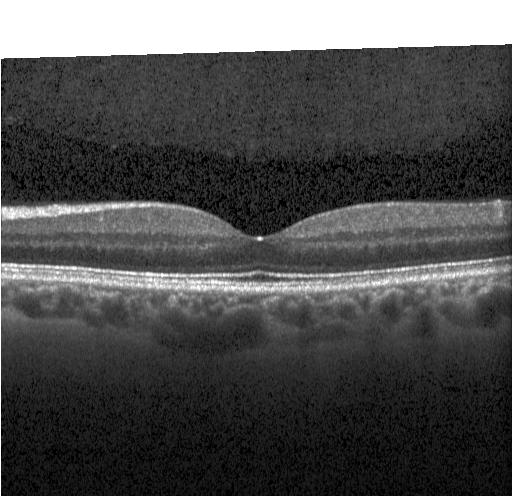

Retinal OCT cross-section — This B-scan demonstrates neither choroidal neovascularization, diabetic macular edema, nor drusen.